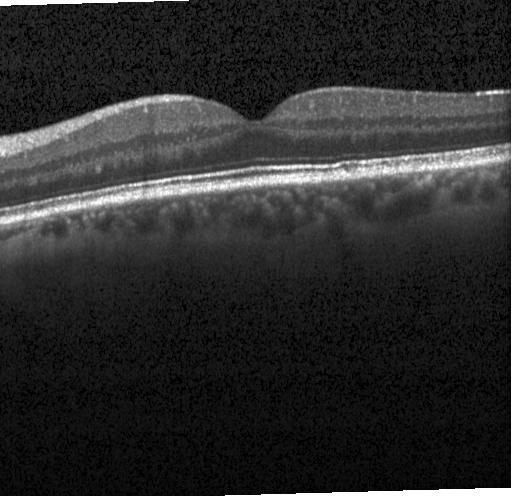
Retinal OCT cross-section. Heidelberg Spectralis. Spectral-domain optical coherence tomography. Through the macula.
The scan shows no evidence of choroidal neovascularization, diabetic macular edema, or drusen.